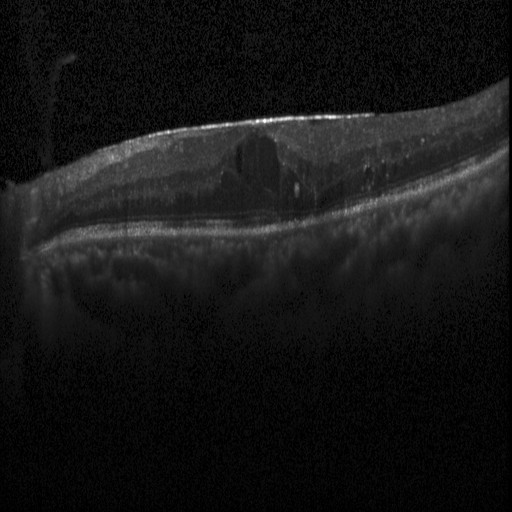 Macular OCT: DME.